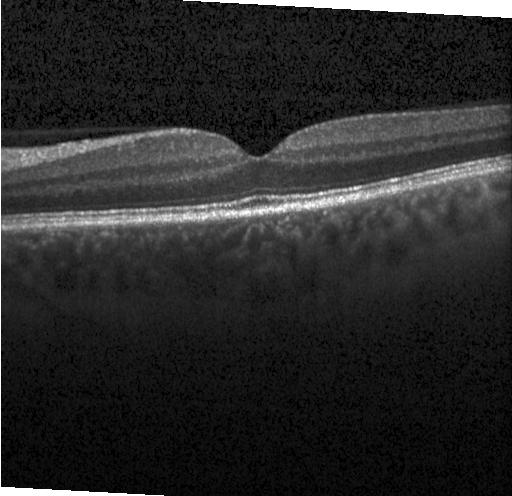
OCT B-scan, spectral-domain optical coherence tomography. Macular OCT: no evidence of CNV, DME, or drusen.